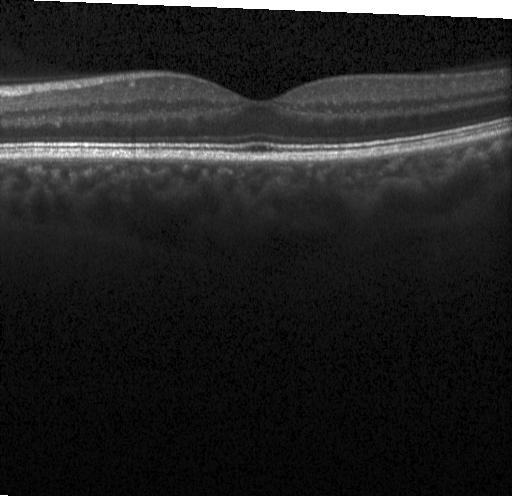
Impression: neither choroidal neovascularization, diabetic macular edema, nor drusen.